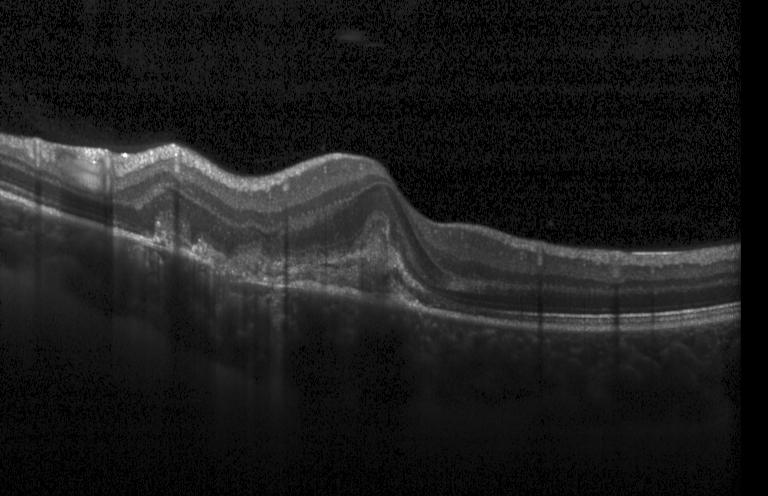

Retinal OCT cross-section showing CNV.